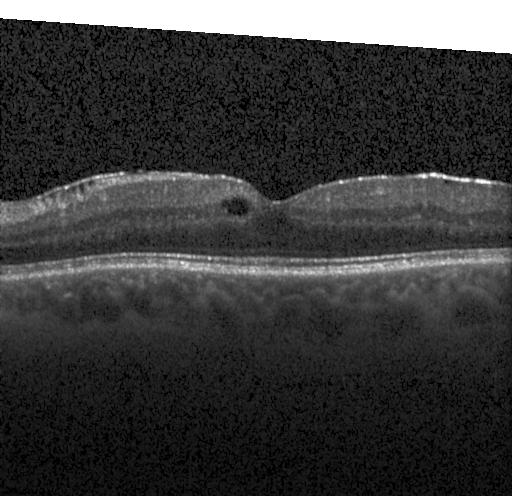 The scan shows diabetic macular edema (DME).